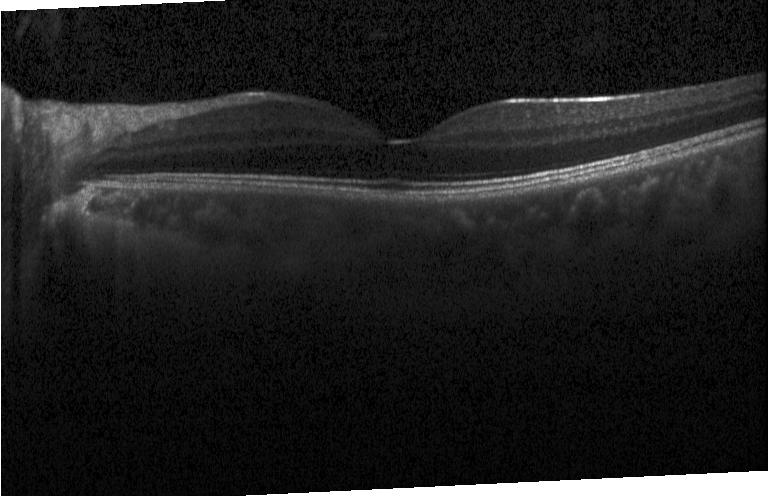

OCT B-scan; instrument: Heidelberg Spectralis — Macular OCT: no evidence of CNV, DME, or drusen.